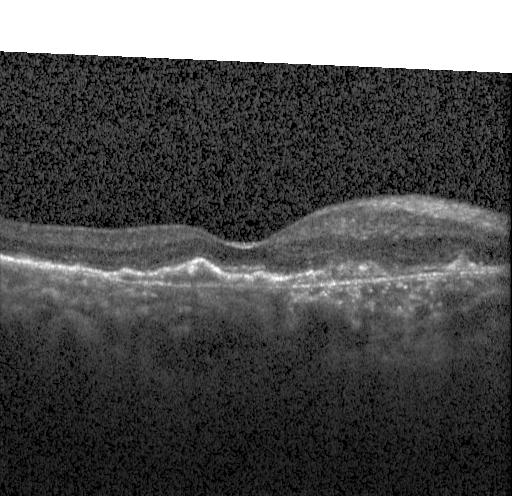
The scan shows choroidal neovascularization.